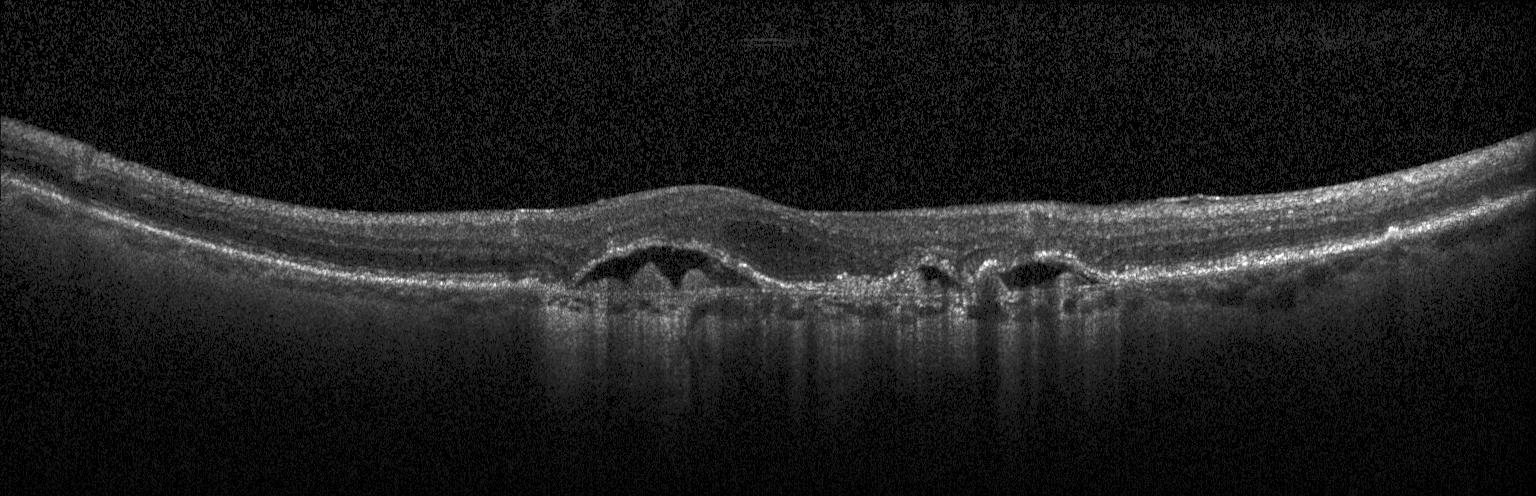 OCT scan showing a choroidal neovascular membrane.